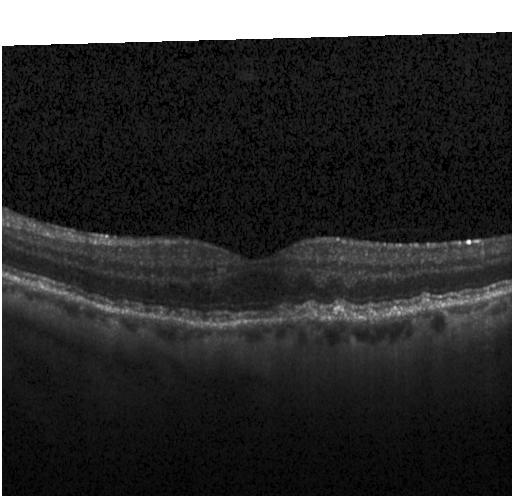 This B-scan demonstrates drusen.